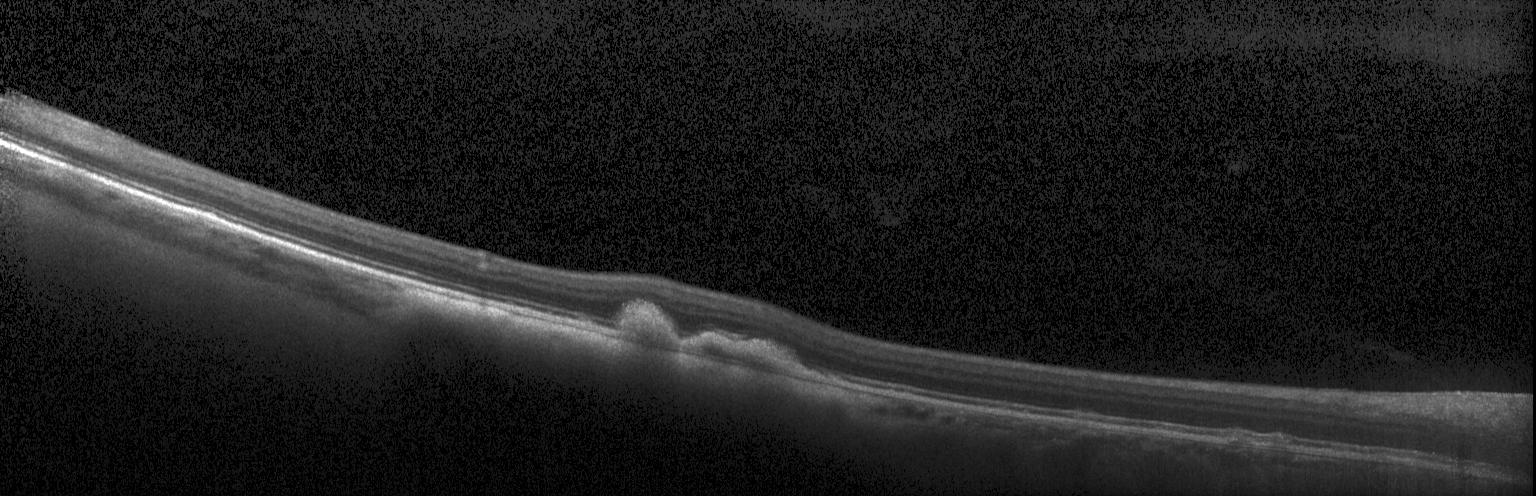 Impression: CNV.